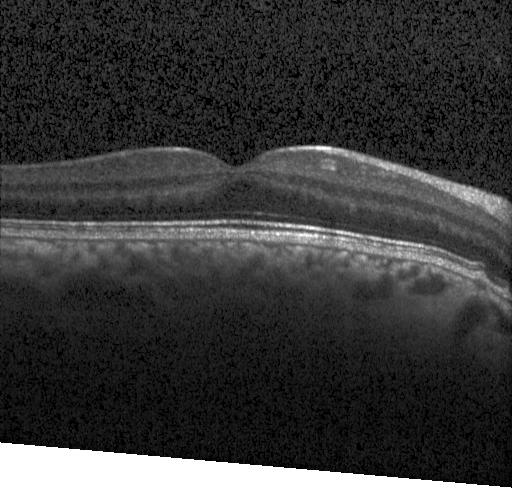
OCT finding: neither CNV, DME, nor drusen.